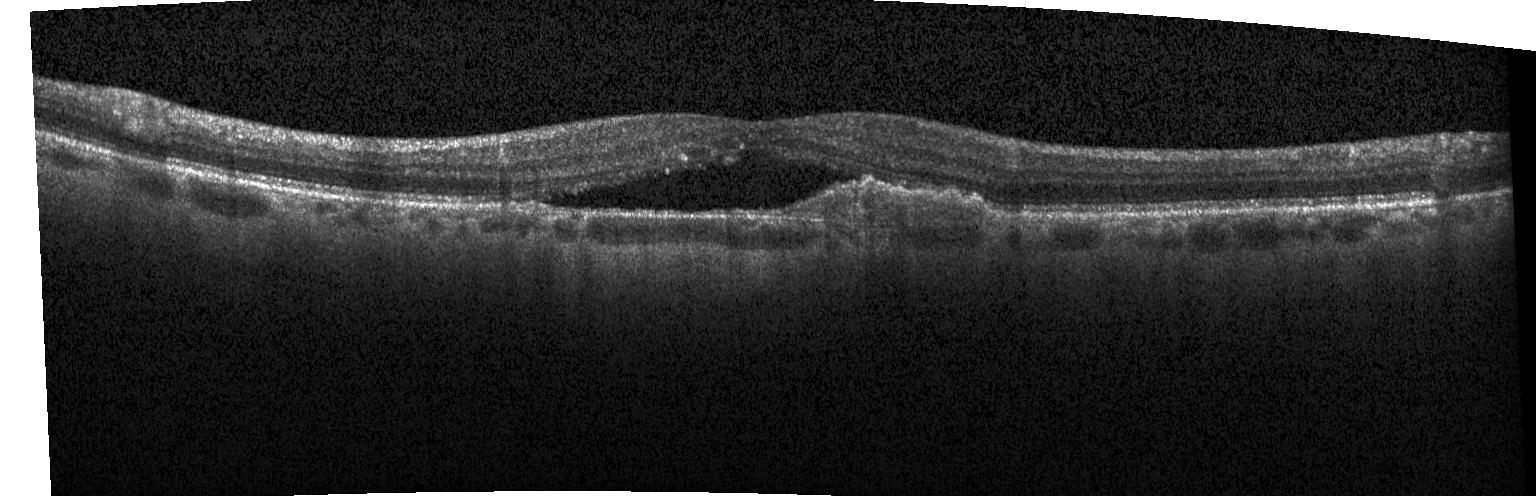
Optical coherence tomography B-scan
A choroidal neovascular membrane.